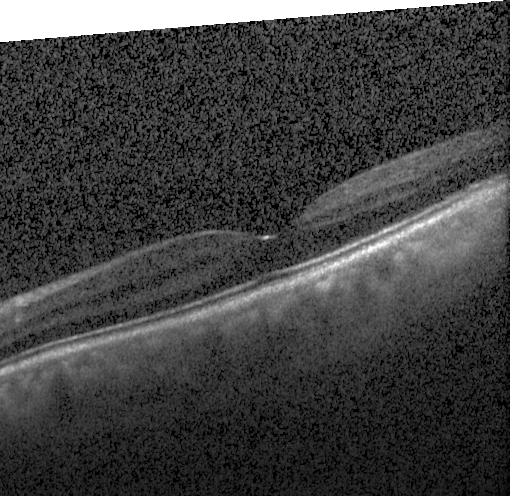 Finding: no evidence of choroidal neovascularization, diabetic macular edema, or drusen.